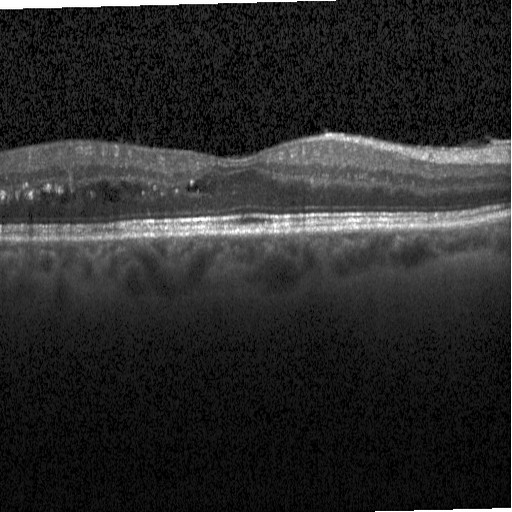 Optical coherence tomography B-scan, centered on the fovea. Finding: diabetic macular edema.